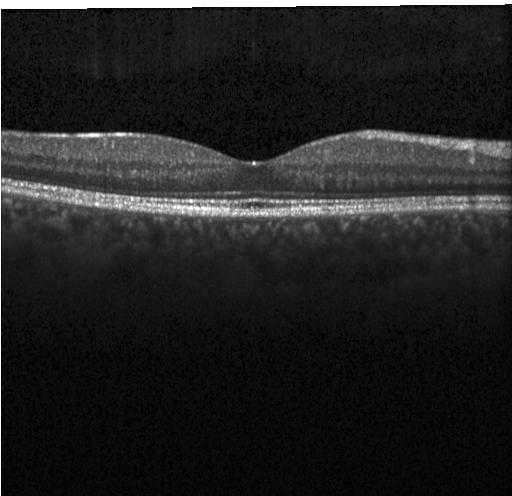 Instrument: Heidelberg Spectralis, spectral-domain optical coherence tomography, fovea-centered, retinal OCT B-scan.
Diagnosis: no evidence of choroidal neovascularization, diabetic macular edema, or drusen.